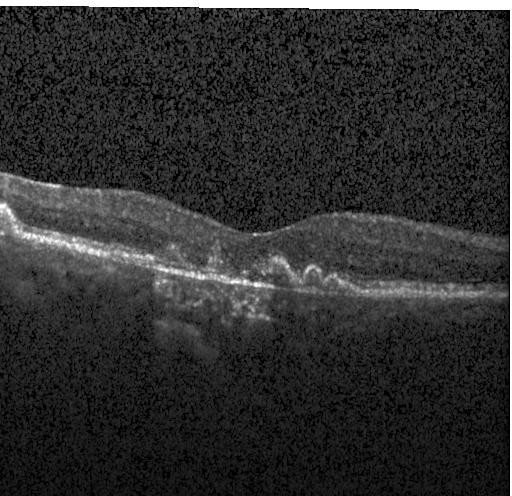

Optical coherence tomography scan; Heidelberg Spectralis.
Impression: choroidal neovascularization.